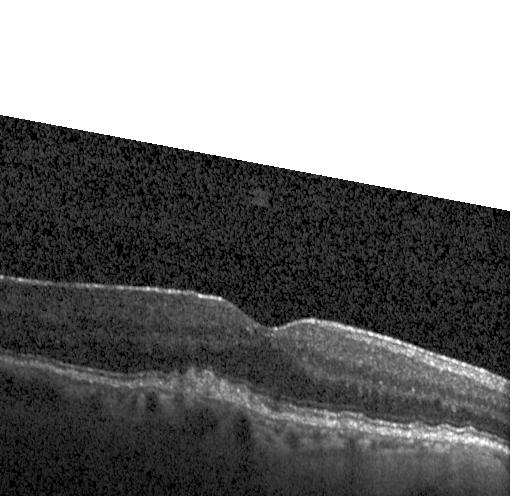 Centered on the fovea, Heidelberg Spectralis OCT system, OCT line scan, SD-OCT. Impression: sub-RPE drusenoid deposits.